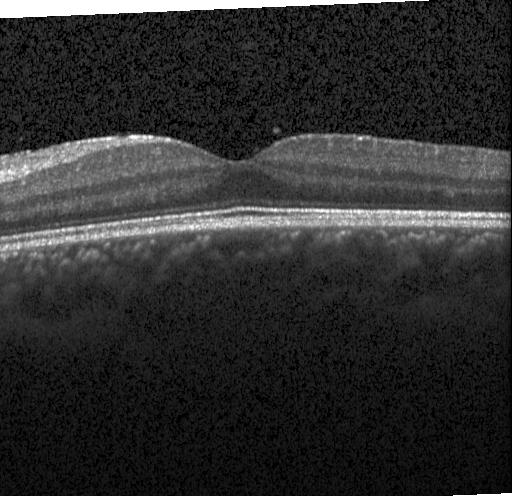 OCT B-scan; centered on the fovea.
Diagnosis: no choroidal neovascularization, diabetic macular edema, or drusen.